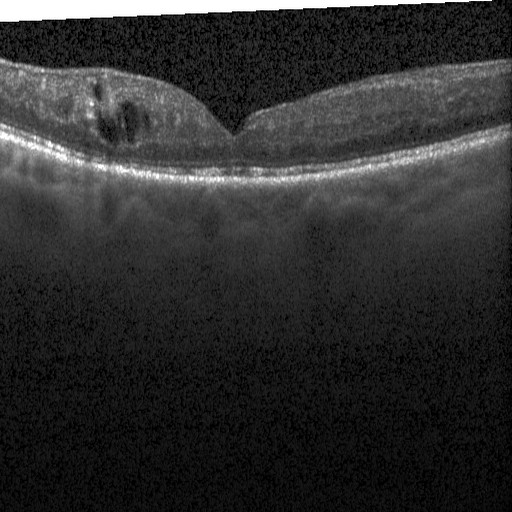

SD-OCT, Heidelberg Spectralis, OCT line scan
Impression: DME.